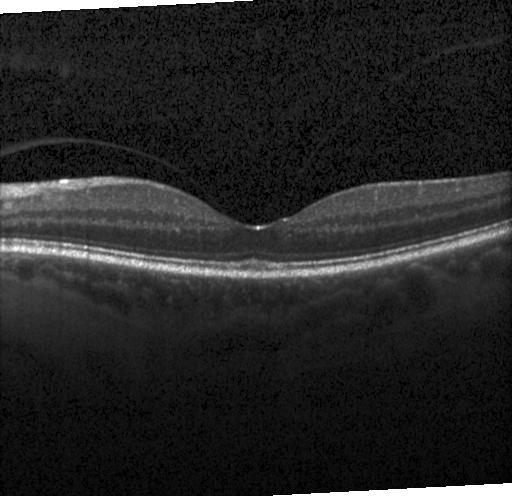

Finding: no evidence of CNV, DME, or drusen.